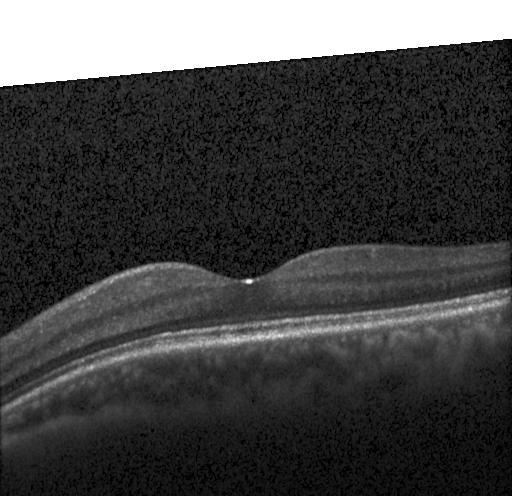 Instrument: Heidelberg Spectralis, fovea-centered, optical coherence tomography scan, SD-OCT.
Macular OCT: no choroidal neovascularization, no diabetic macular edema, and no drusen.